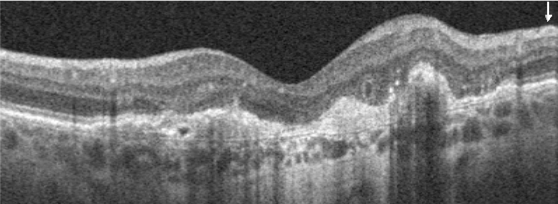
Assessment: AMD.